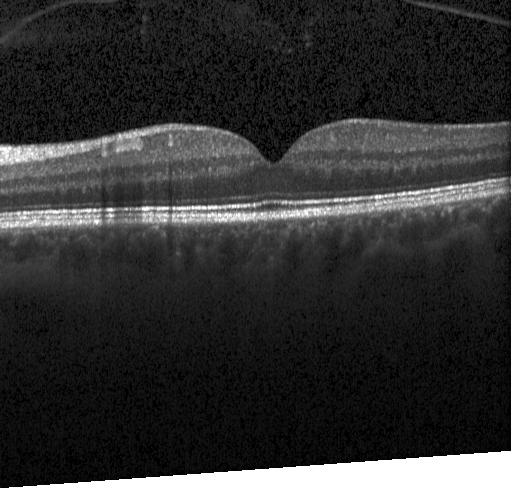 Optical coherence tomography B-scan; SD-OCT; Heidelberg Spectralis OCT system; horizontal scan through the fovea
OCT finding: neither CNV, DME, nor drusen.